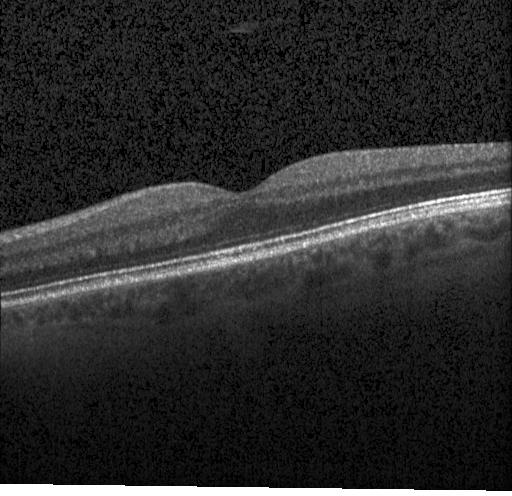
Optical coherence tomography B-scan. Acquired on a Heidelberg Spectralis. Fovea-centered. Impression: no choroidal neovascularization, diabetic macular edema, or drusen.